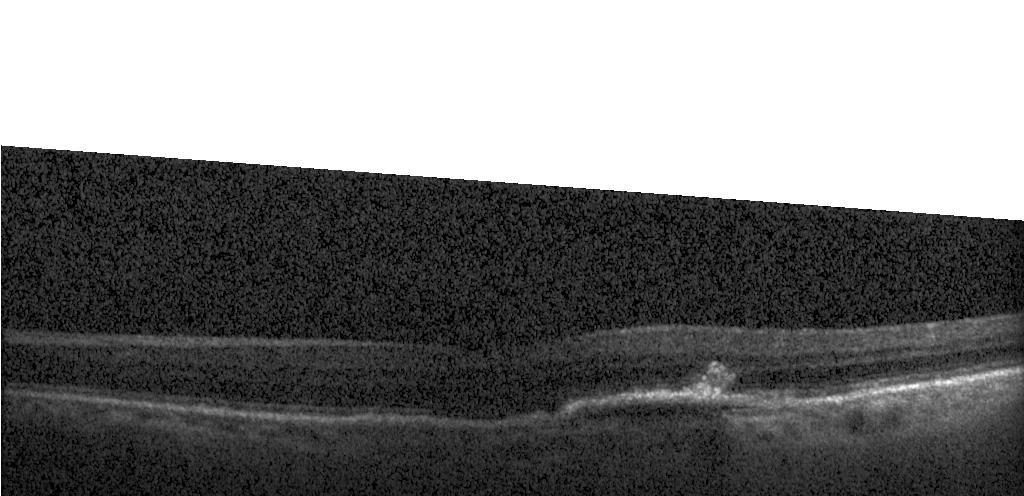

OCT line scan — Finding: CNV.